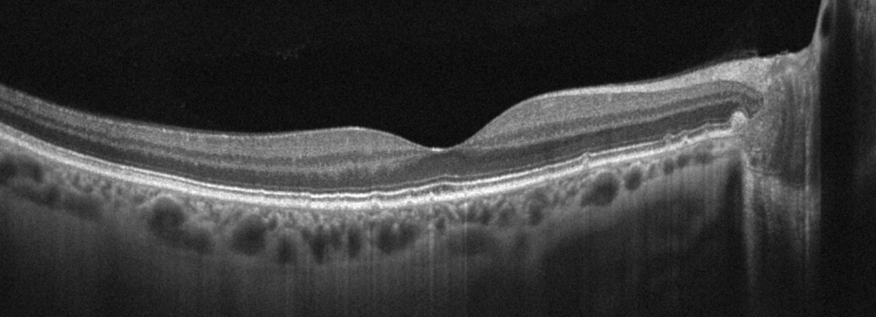 OCT B-scan. OCT finding: age-related macular degeneration (AMD).